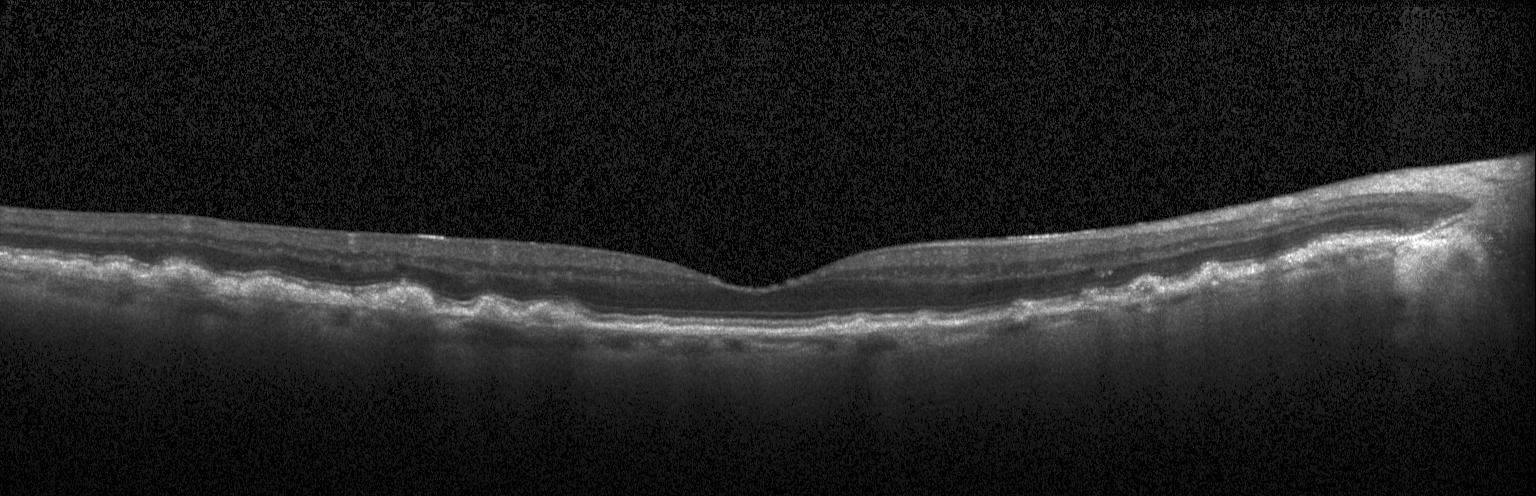 Acquired on a Heidelberg Spectralis. Horizontal scan through the fovea. Optical coherence tomography B-scan. SD-OCT.
Finding: multiple drusen.